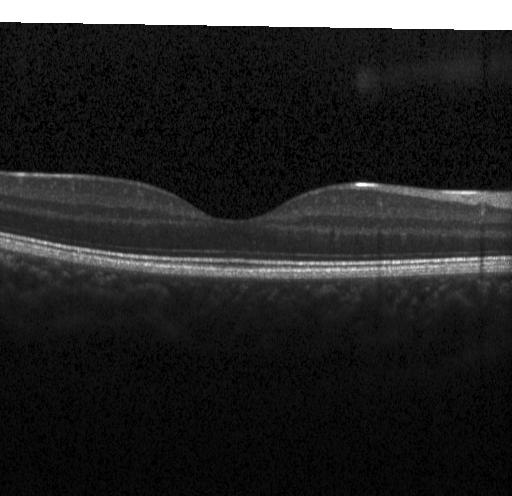 Heidelberg Spectralis OCT system. Spectral-domain OCT. Retinal OCT B-scan. Centered on the fovea — OCT finding: no CNV, no DME, and no drusen.